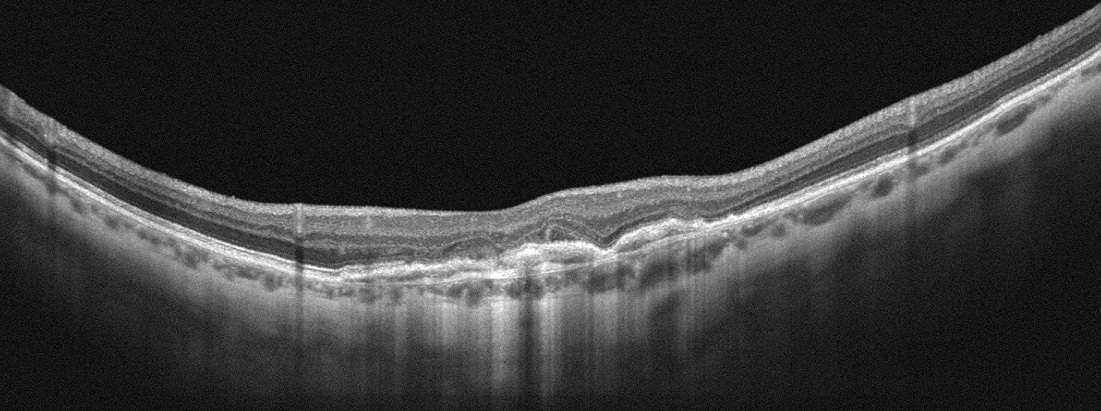

Macular scan; retinal OCT cross-section — Dx: age-related macular degeneration.